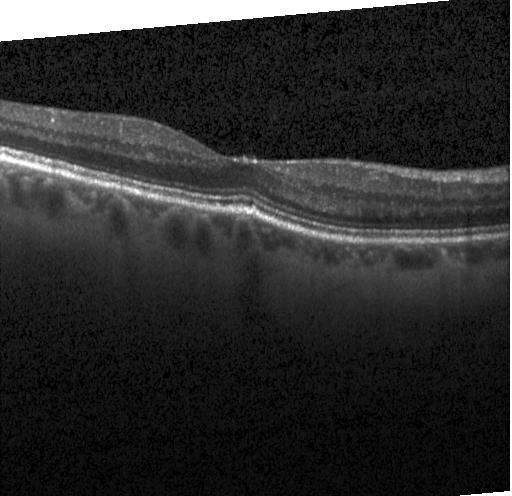
Through the macula, spectral-domain optical coherence tomography, optical coherence tomography B-scan, instrument: Heidelberg Spectralis. Assessment: neither choroidal neovascularization, diabetic macular edema, nor drusen.